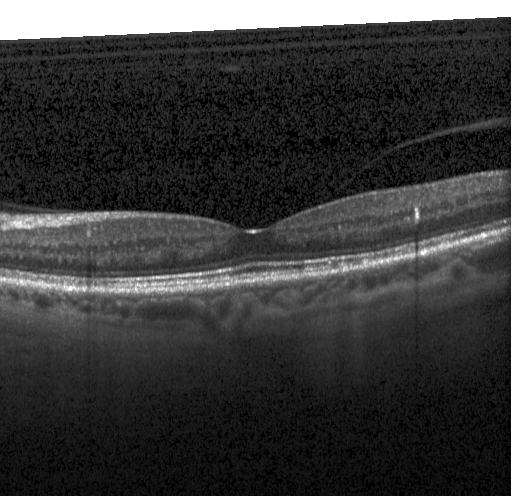 Heidelberg Spectralis · spectral-domain OCT · optical coherence tomography scan.
Finding: neither CNV, DME, nor drusen.